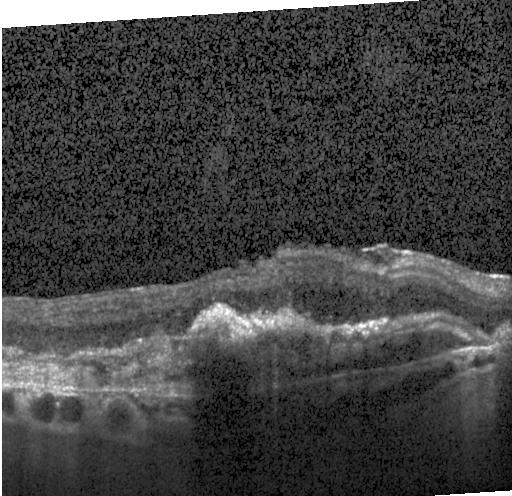 Macular OCT demonstrating CNV.